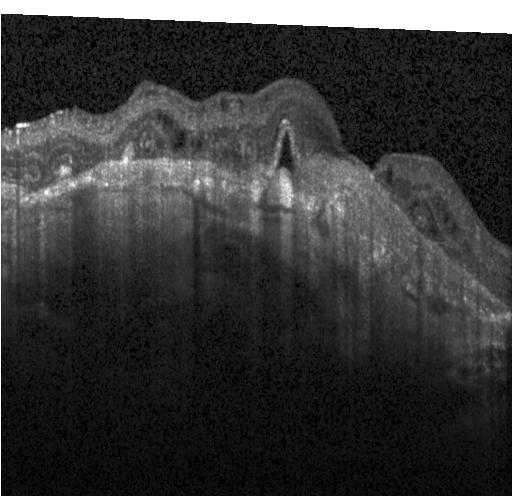 Macular OCT demonstrating CNV.